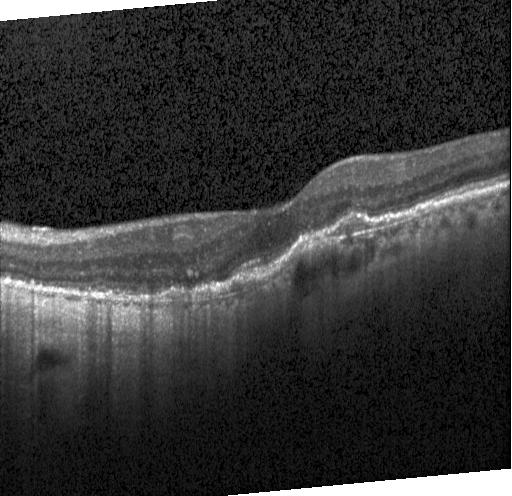

Macular OCT demonstrating choroidal neovascularization.